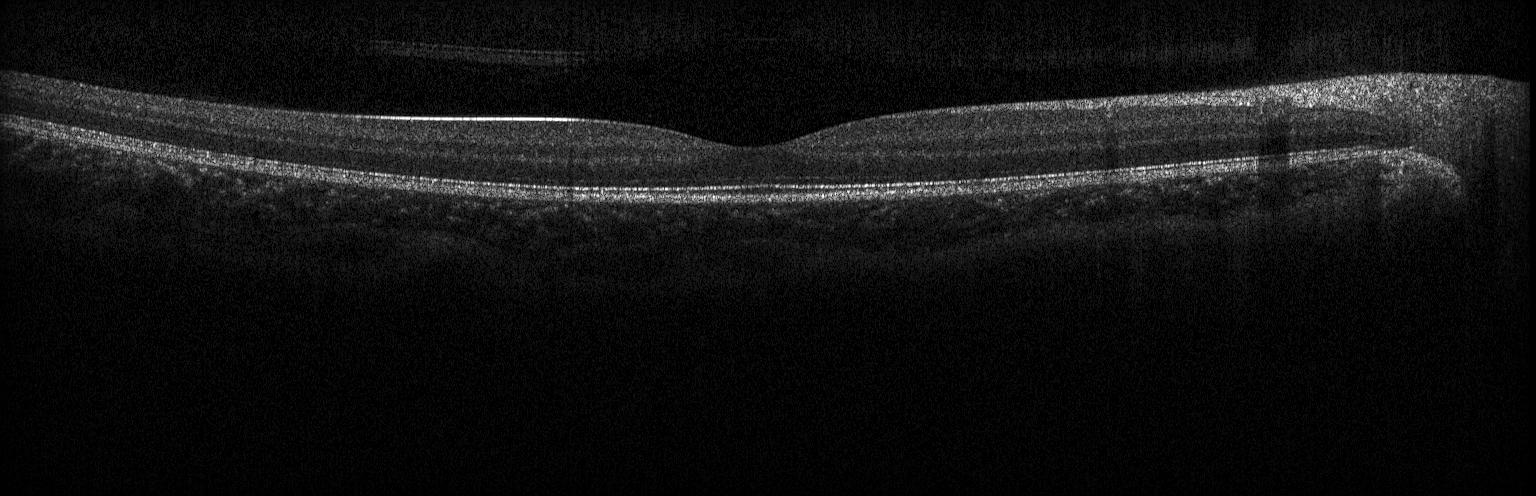

Macular scan, OCT B-scan, SD-OCT, instrument: Heidelberg Spectralis — This B-scan demonstrates neither choroidal neovascularization, diabetic macular edema, nor drusen.